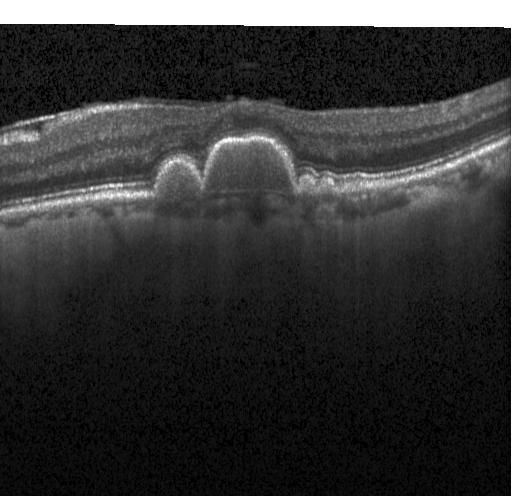 Heidelberg Spectralis. Retinal OCT cross-section. Spectral-domain OCT. Fovea-centered. Finding: a choroidal neovascular membrane.